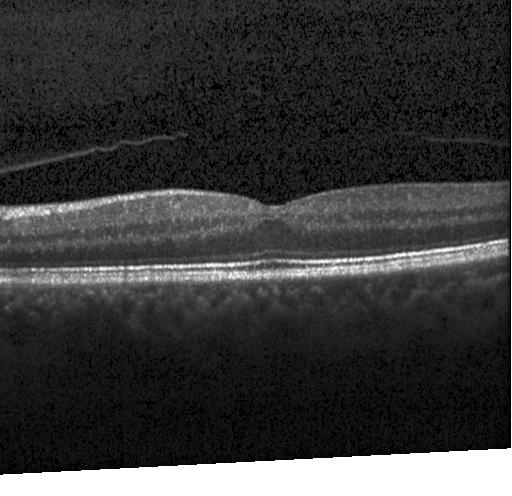
This B-scan demonstrates no choroidal neovascularization, no diabetic macular edema, and no drusen.